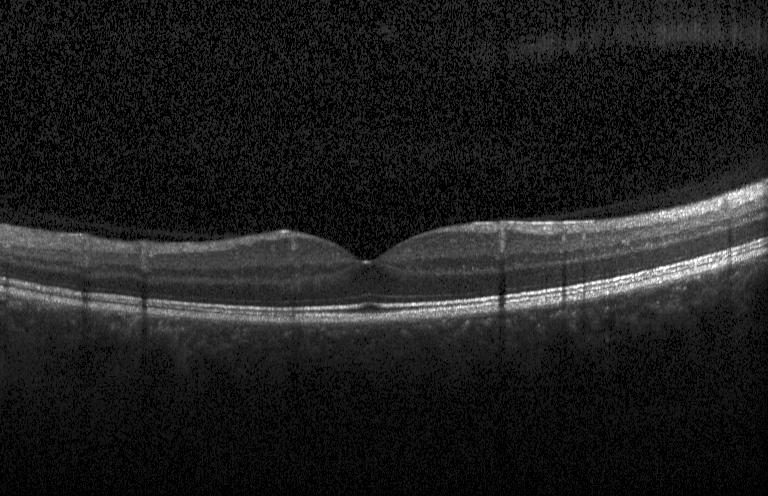
Spectral-domain OCT B-scan: no choroidal neovascularization, diabetic macular edema, or drusen.